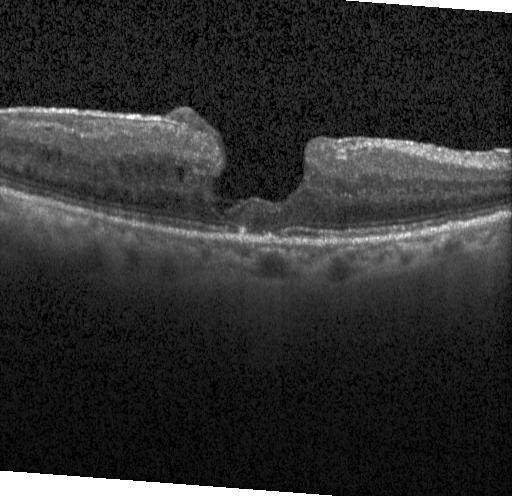
Diagnosis: diabetic macular edema.